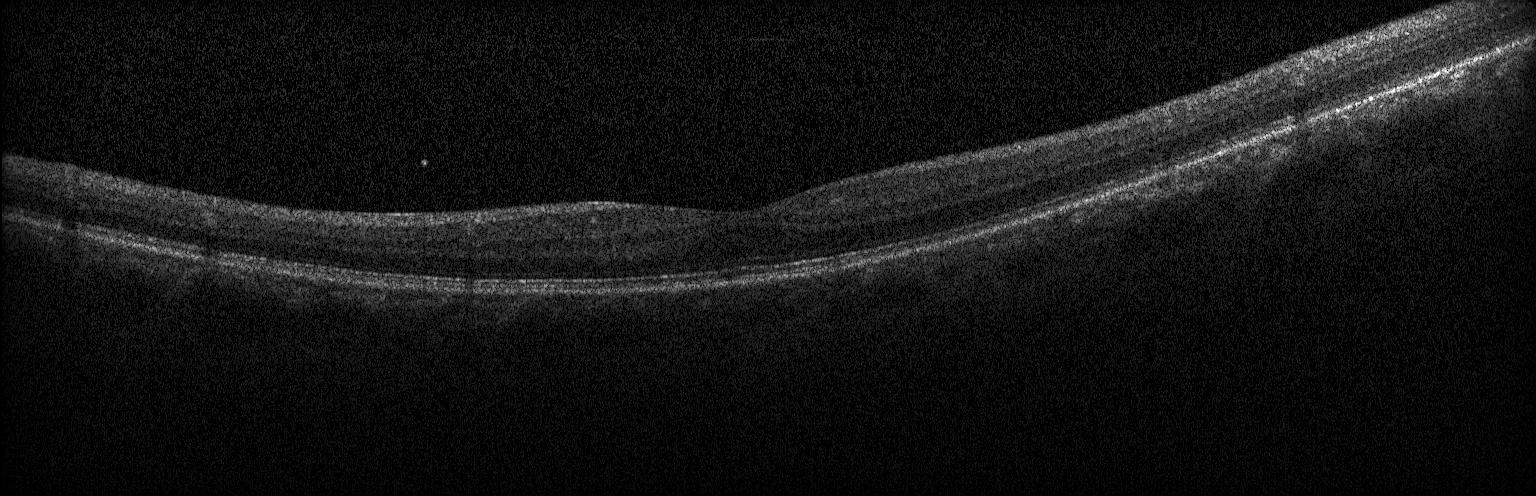

OCT B-scan
Dx: neither choroidal neovascularization, diabetic macular edema, nor drusen.